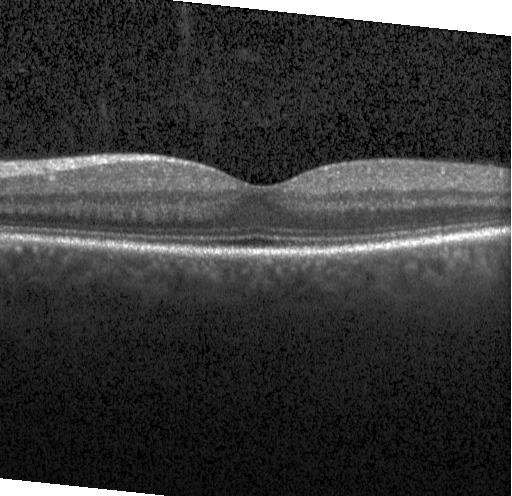 Spectral-domain OCT · optical coherence tomography B-scan · horizontal scan through the fovea · Heidelberg Spectralis OCT system — Impression: no choroidal neovascularization, diabetic macular edema, or drusen.